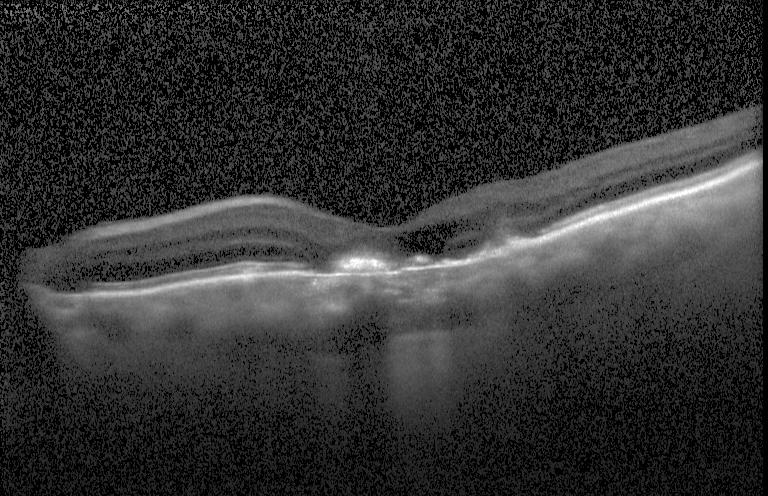 Impression: choroidal neovascularization (CNV).